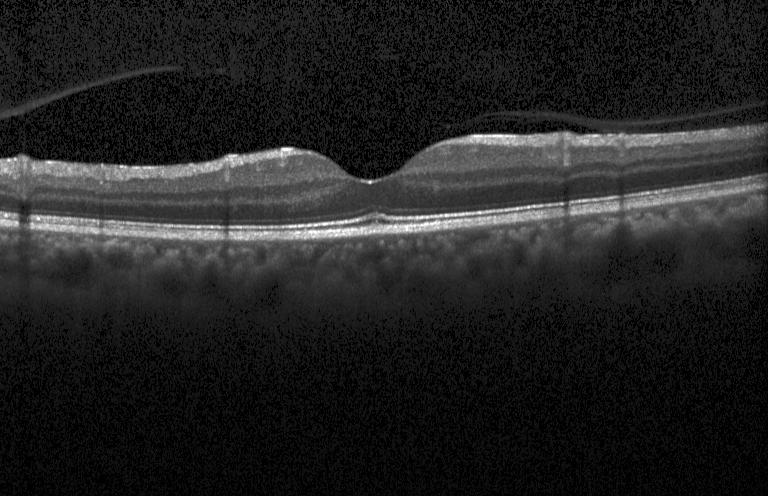

Dx: no choroidal neovascularization, no diabetic macular edema, and no drusen.